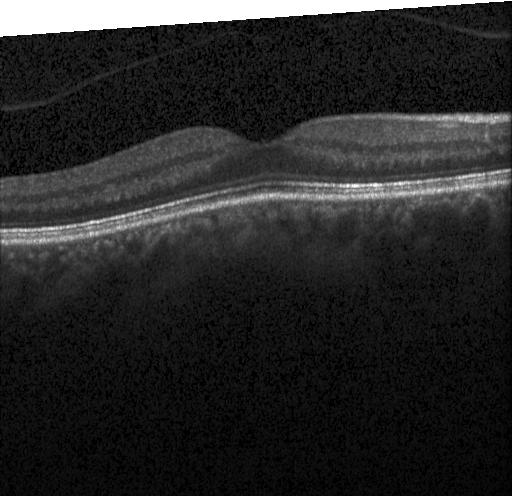 Spectral-domain optical coherence tomography, optical coherence tomography scan, centered on the fovea. Impression: no CNV, no DME, and no drusen.